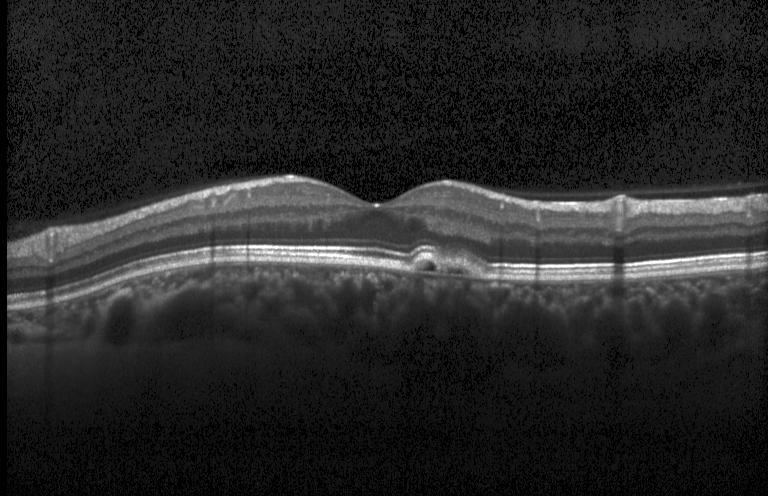 SD-OCT, OCT B-scan, centered on the fovea, Heidelberg Spectralis
Finding: a choroidal neovascular membrane.